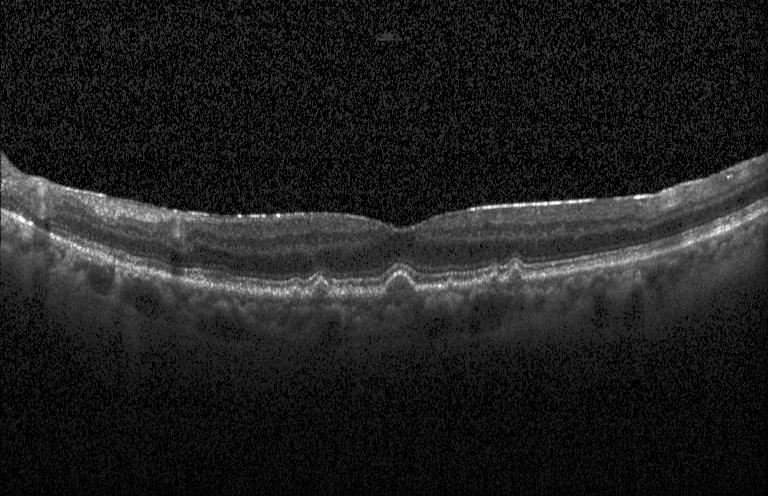
Finding: multiple drusen.